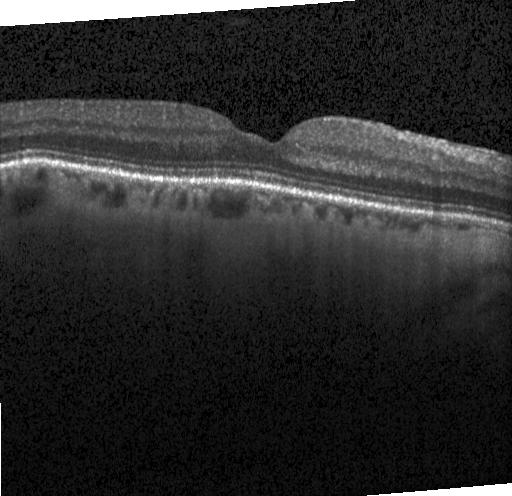 Fovea-centered; Heidelberg Spectralis OCT system; retinal OCT B-scan; spectral-domain OCT
Finding: no CNV, DME, or drusen.